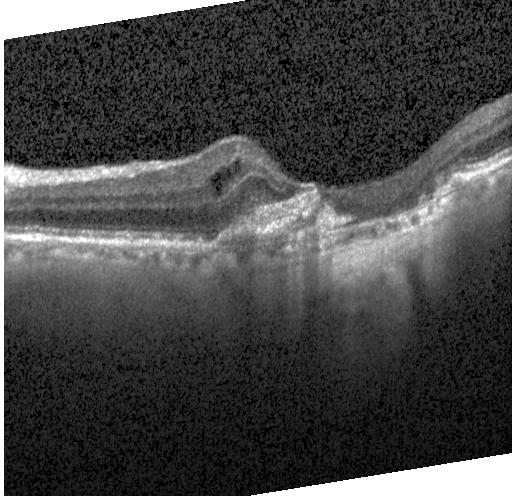

Impression: CNV.